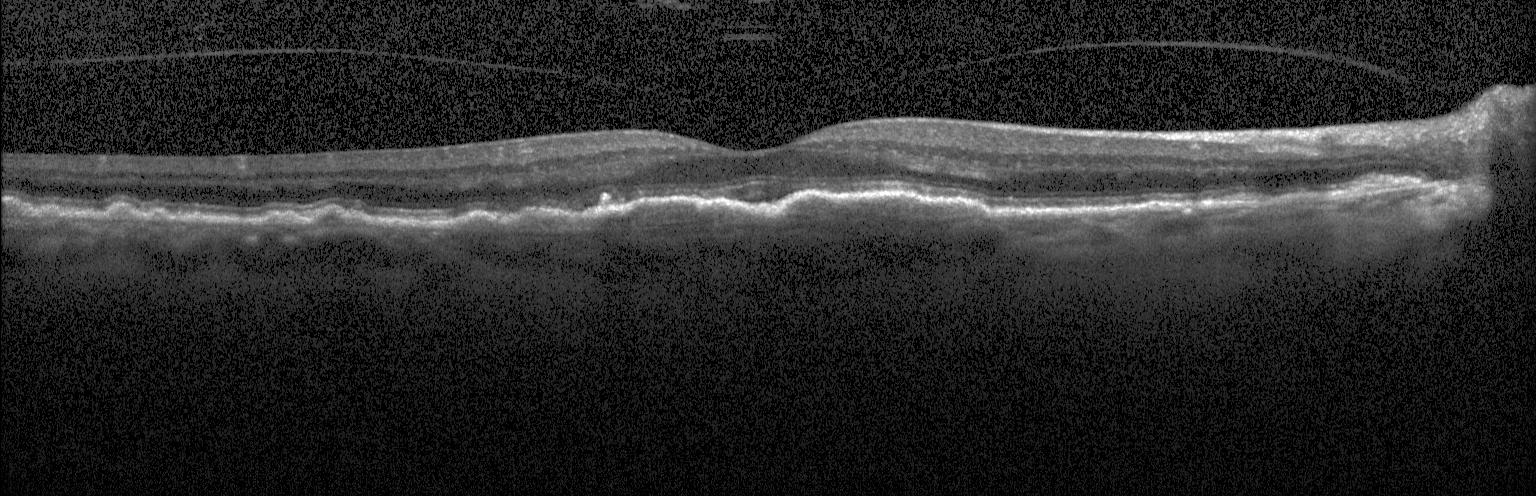 Macular OCT demonstrating a choroidal neovascular membrane.